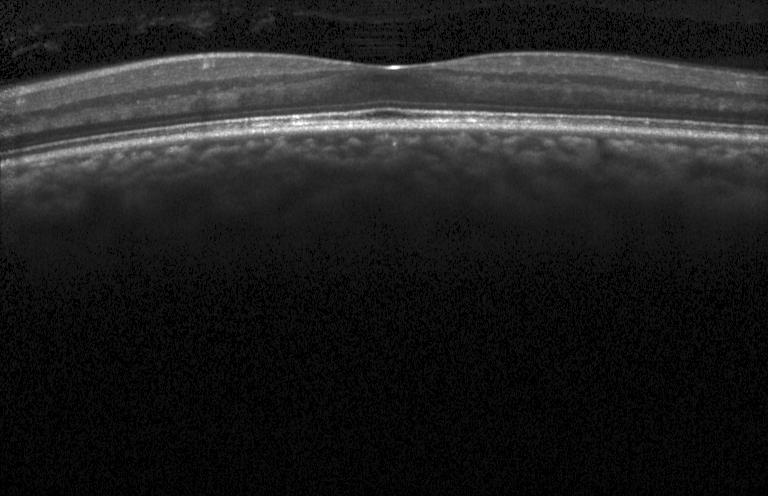

Instrument: Heidelberg Spectralis, OCT line scan, horizontal scan through the fovea.
Impression: no choroidal neovascularization, no diabetic macular edema, and no drusen.